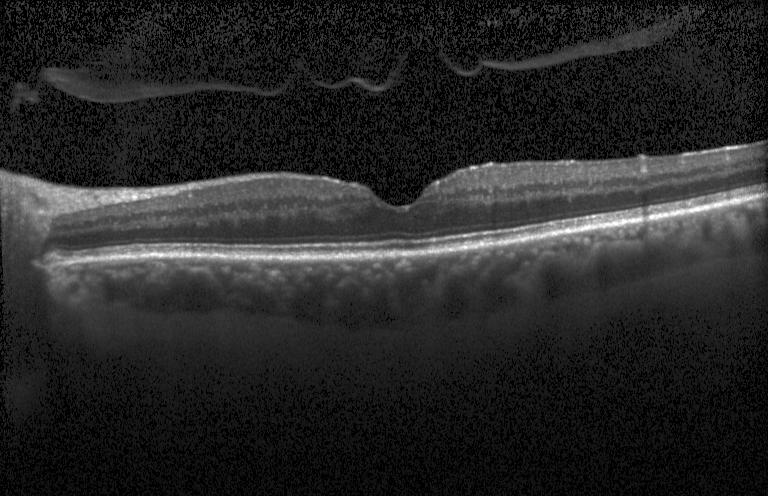

Retinal OCT cross-section showing neither CNV, DME, nor drusen.